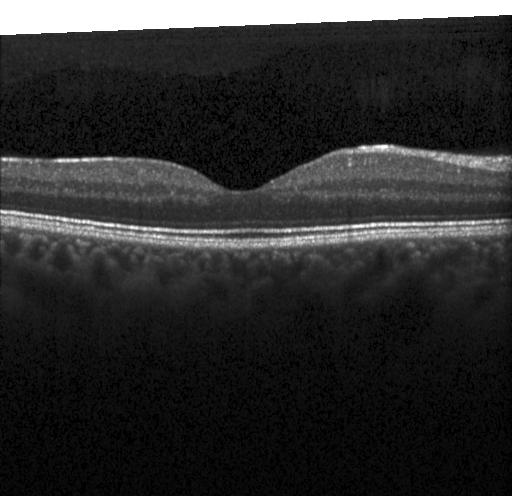 Spectral-domain OCT · Heidelberg Spectralis OCT system · OCT B-scan — This B-scan demonstrates no choroidal neovascularization, diabetic macular edema, or drusen.